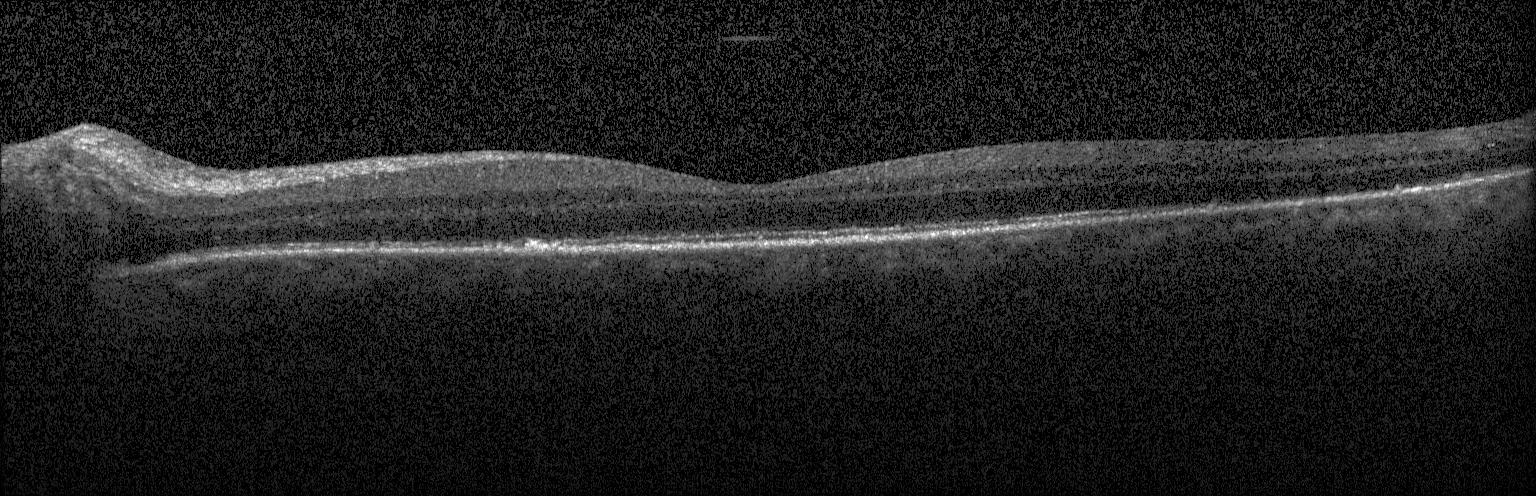 SD-OCT · optical coherence tomography B-scan · instrument: Heidelberg Spectralis
Macular OCT: no CNV, no DME, and no drusen.